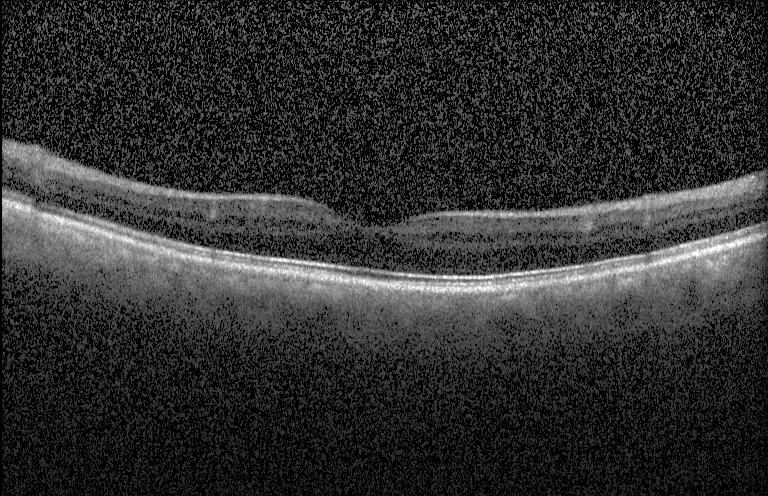

Diagnosis: neither CNV, DME, nor drusen.